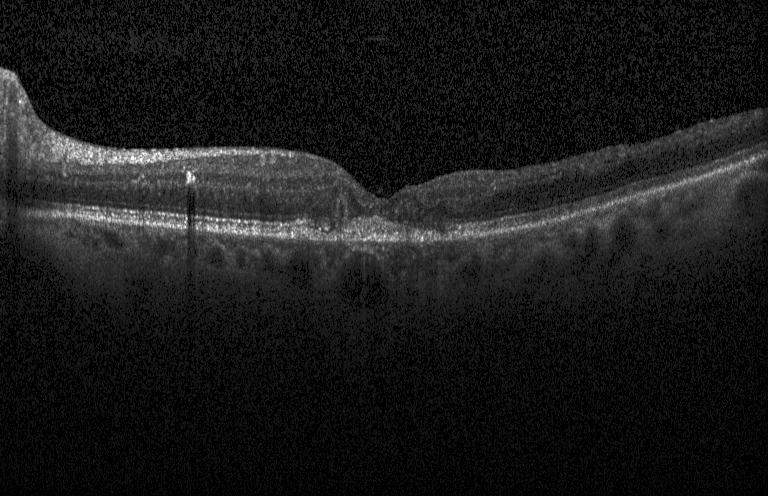

Finding: a choroidal neovascular membrane.